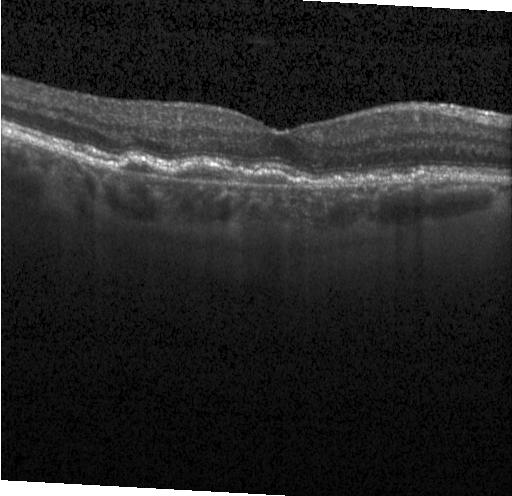

Heidelberg Spectralis, fovea-centered, OCT line scan
OCT finding: CNV.